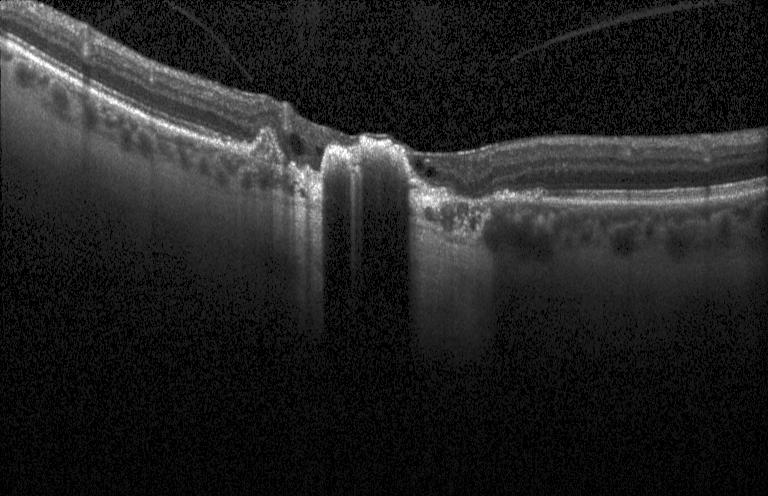
Retinal OCT cross-section showing a choroidal neovascular membrane.